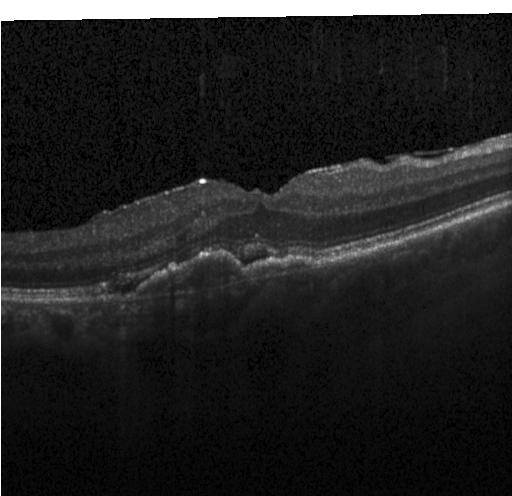 Diagnosis: choroidal neovascularization (CNV).